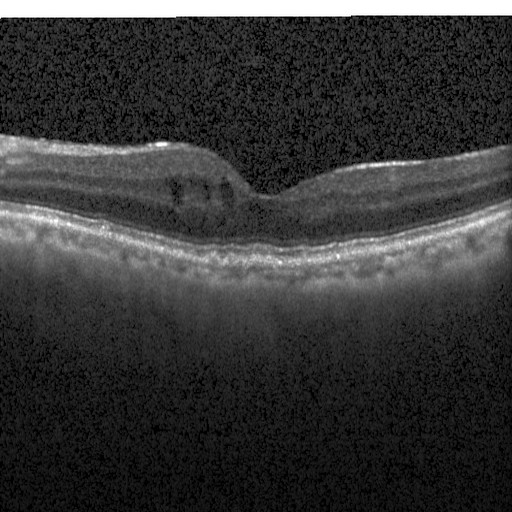 Diagnosis: DME.